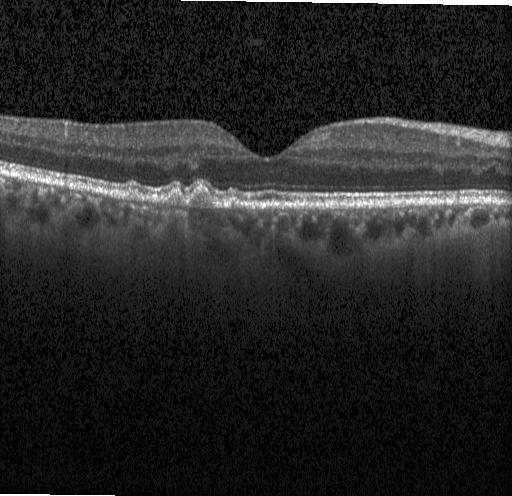 Finding: sub-RPE drusenoid deposits.